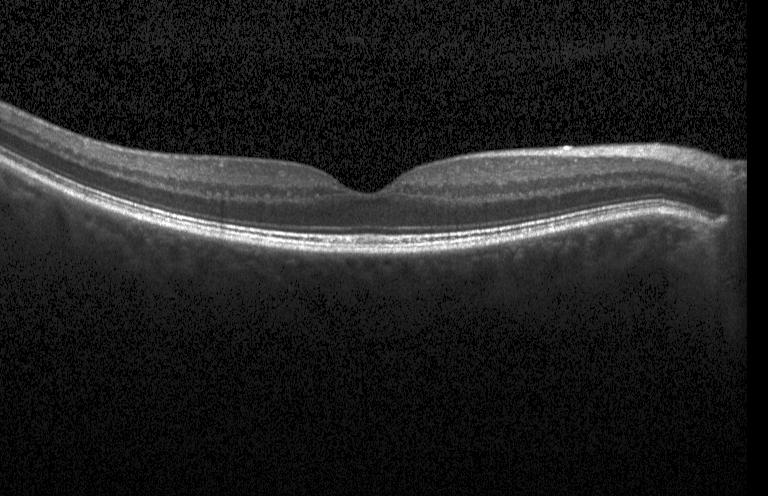 Retinal OCT B-scan, spectral-domain OCT
The scan shows no choroidal neovascularization, diabetic macular edema, or drusen.